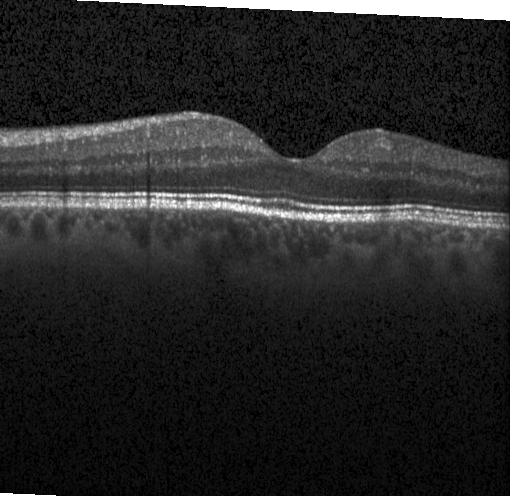

OCT B-scan showing no evidence of CNV, DME, or drusen.